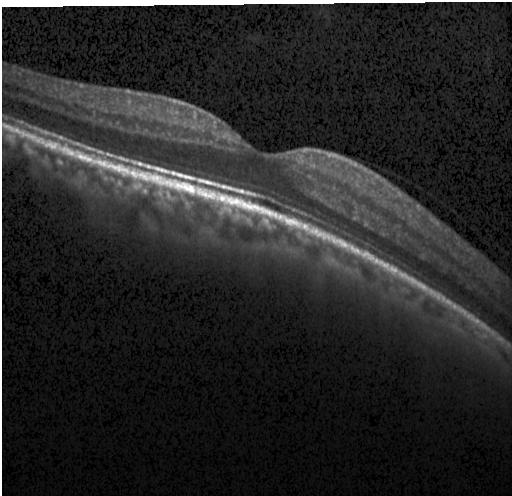 OCT B-scan; horizontal scan through the fovea. Diagnosis: no CNV, DME, or drusen.